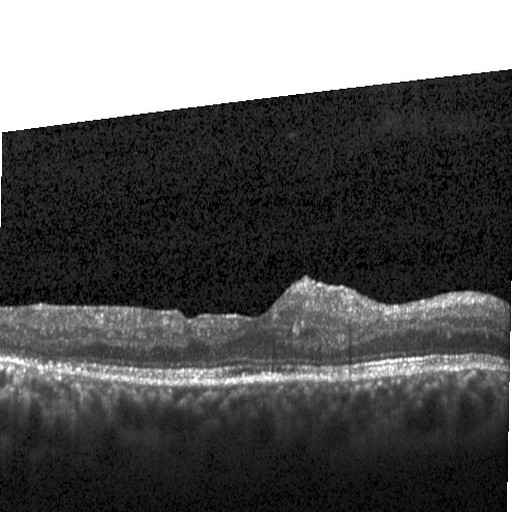

Macular OCT: diabetic macular edema (DME).